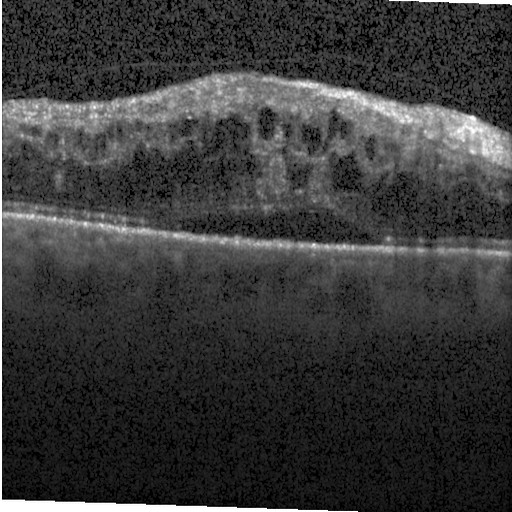 Centered on the fovea. OCT line scan. Heidelberg Spectralis
Diagnosis: diabetic macular edema.